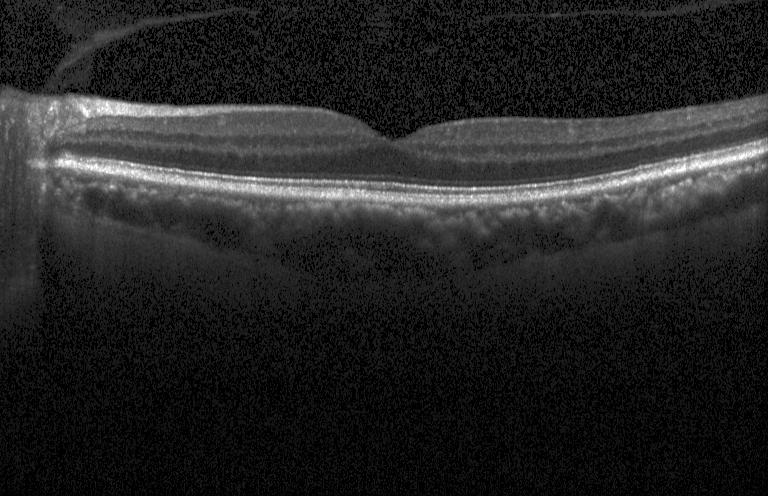
SD-OCT; optical coherence tomography B-scan; centered on the fovea; Heidelberg Spectralis OCT system. Impression: no evidence of choroidal neovascularization, diabetic macular edema, or drusen.